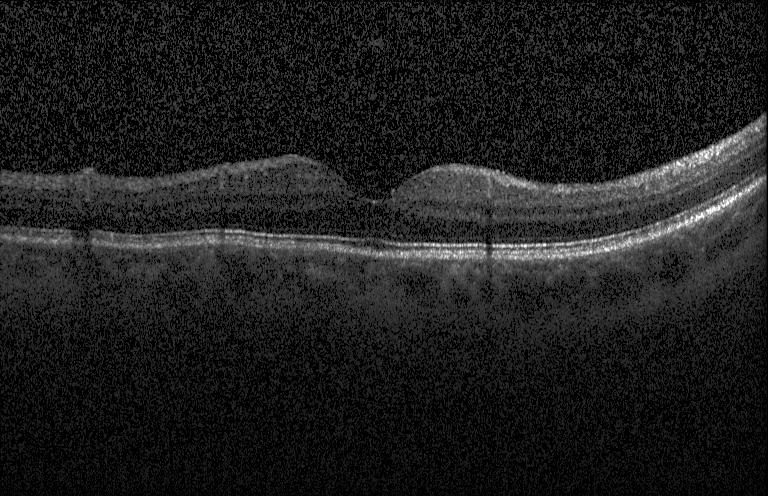

Retinal OCT B-scan; spectral-domain OCT. Assessment: no choroidal neovascularization, diabetic macular edema, or drusen.